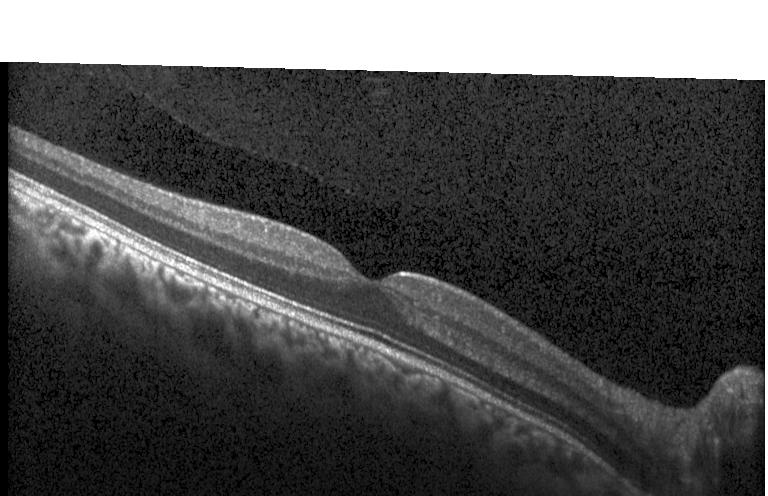 Retinal OCT cross-section showing no choroidal neovascularization, no diabetic macular edema, and no drusen.